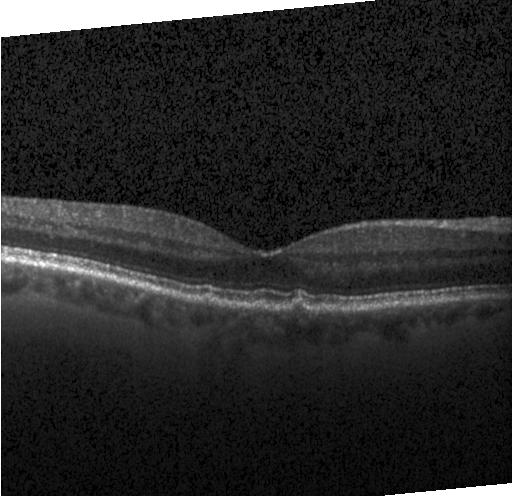
Centered on the fovea, Heidelberg Spectralis OCT system, OCT B-scan. Diagnosis: multiple drusen.